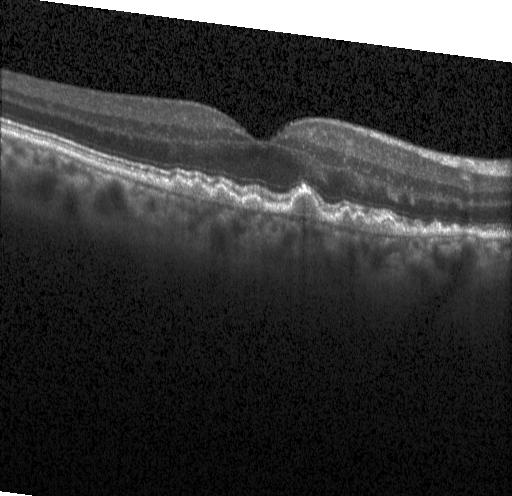
SD-OCT; Heidelberg Spectralis OCT system; centered on the fovea; OCT line scan — Macular OCT: sub-RPE drusenoid deposits.